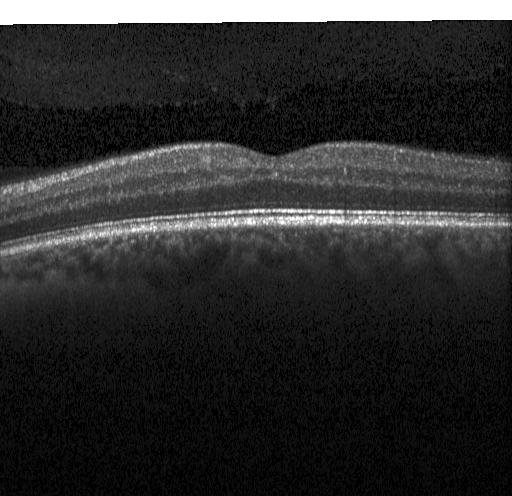
Optical coherence tomography B-scan; Heidelberg Spectralis OCT system; spectral-domain optical coherence tomography; horizontal scan through the fovea
Diagnosis: no choroidal neovascularization, no diabetic macular edema, and no drusen.